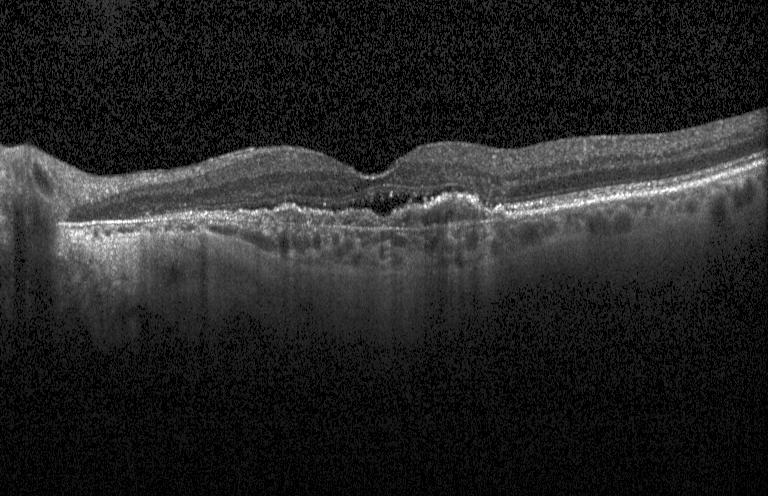

SD-OCT. Through the macula. Retinal OCT B-scan. Instrument: Heidelberg Spectralis. OCT finding: a choroidal neovascular membrane.